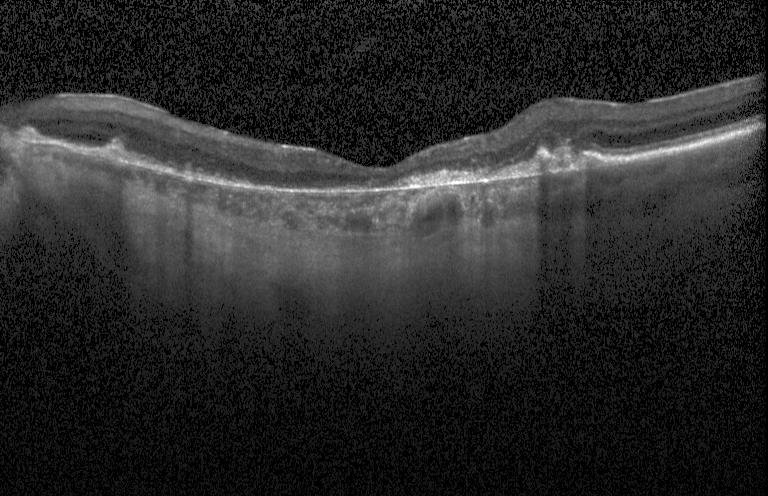

SD-OCT · retinal OCT cross-section · Heidelberg Spectralis OCT system · macular scan
The scan shows a choroidal neovascular membrane.